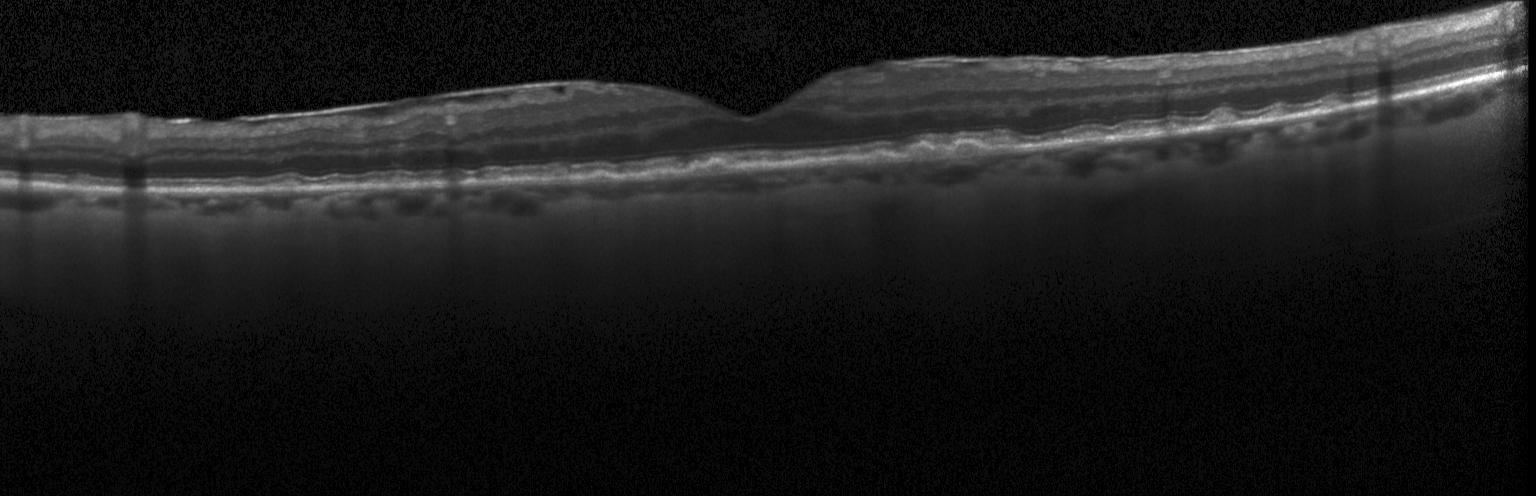

Retinal OCT B-scan — Assessment: drusen.